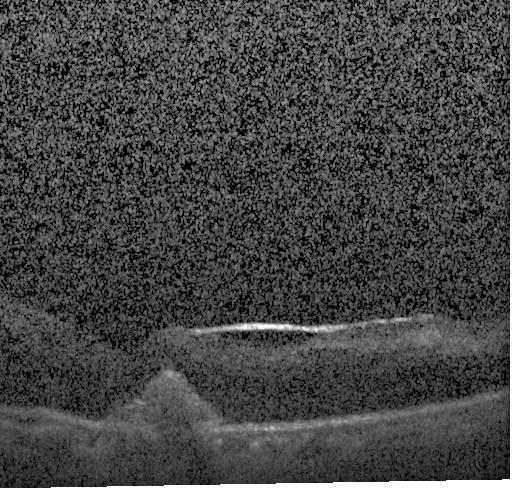
OCT B-scan; instrument: Heidelberg Spectralis; spectral-domain OCT. Assessment: a choroidal neovascular membrane.